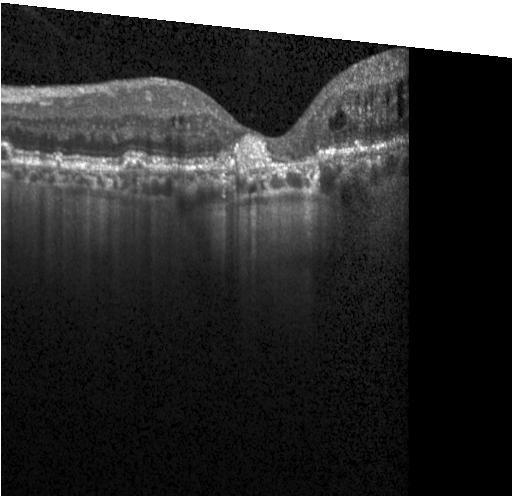

Through the macula · spectral-domain optical coherence tomography · OCT B-scan — Diagnosis: CNV.